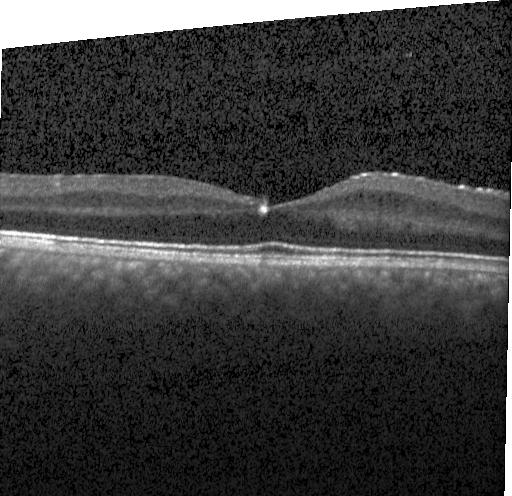
OCT line scan. Fovea-centered — Assessment: diabetic macular edema (DME).